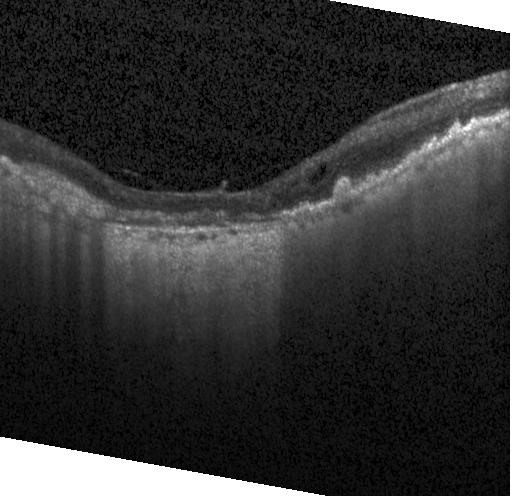
OCT B-scan
This B-scan demonstrates choroidal neovascularization.